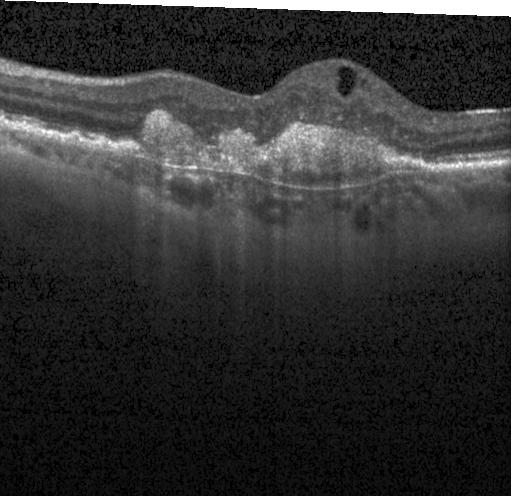
Spectral-domain OCT B-scan: choroidal neovascularization.